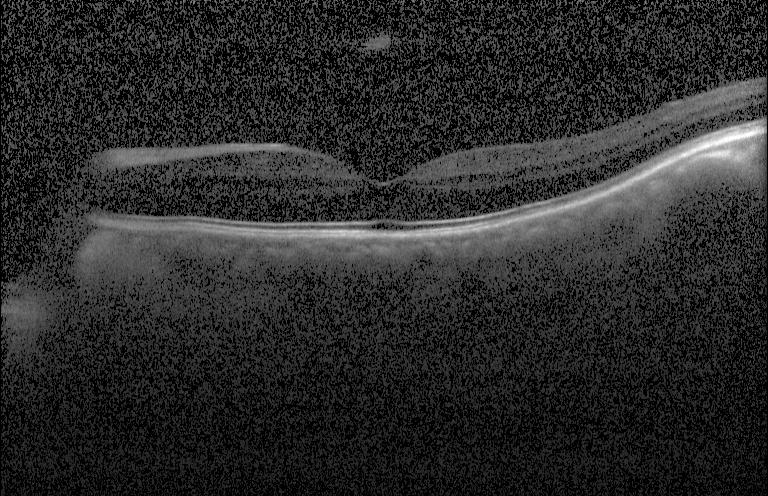
OCT B-scan. Macular OCT: no CNV, DME, or drusen.